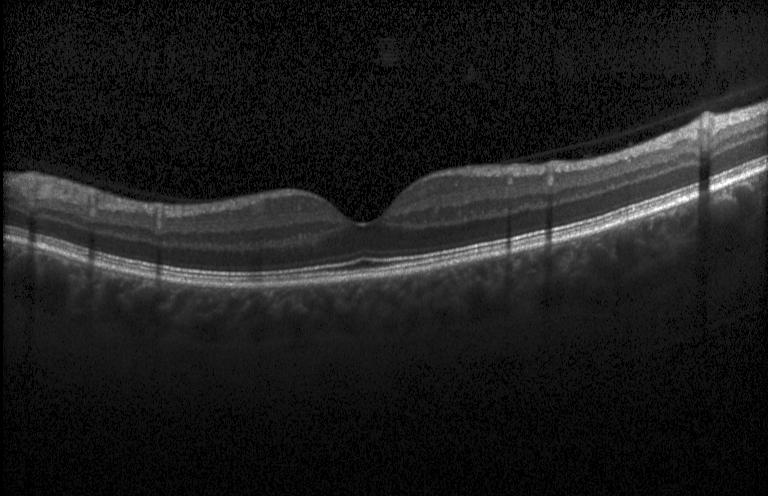 OCT B-scan. Impression: neither choroidal neovascularization, diabetic macular edema, nor drusen.